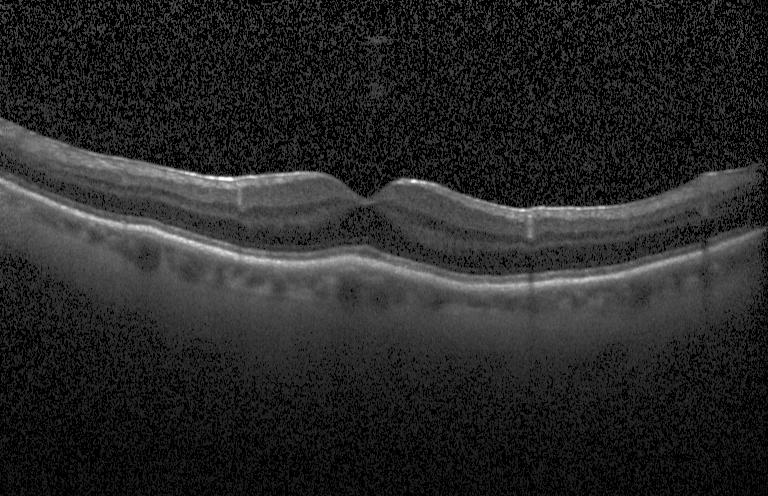
Spectral-domain OCT B-scan: no evidence of choroidal neovascularization, diabetic macular edema, or drusen.